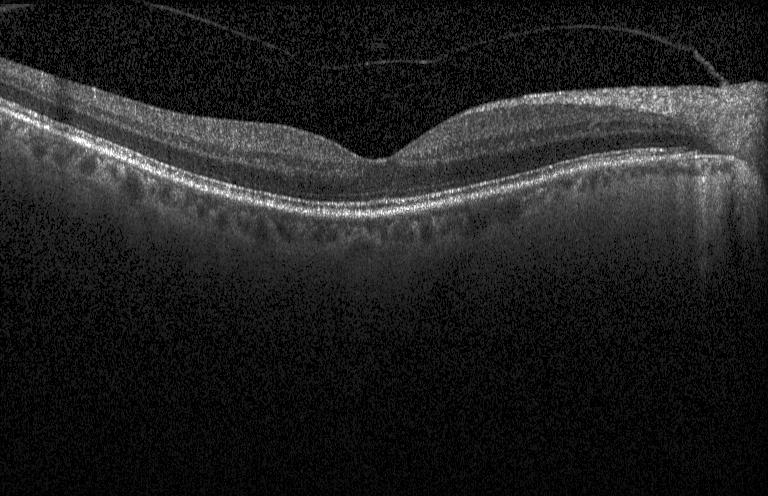
OCT B-scan, SD-OCT
Neither choroidal neovascularization, diabetic macular edema, nor drusen.